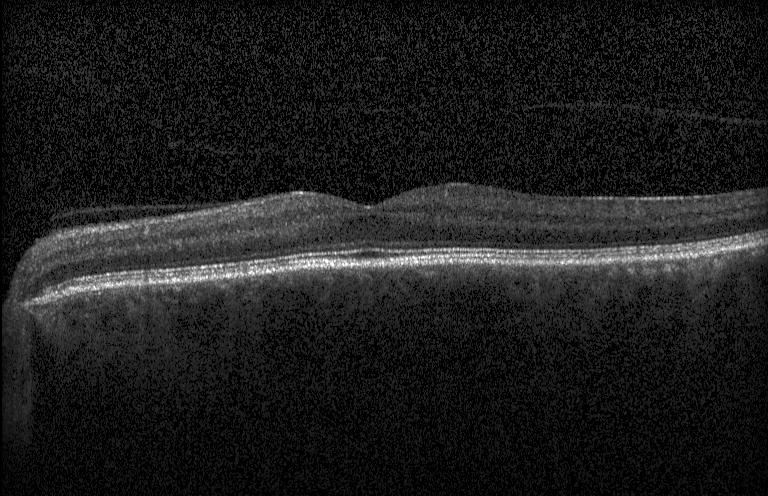 Diagnosis: no evidence of CNV, DME, or drusen.